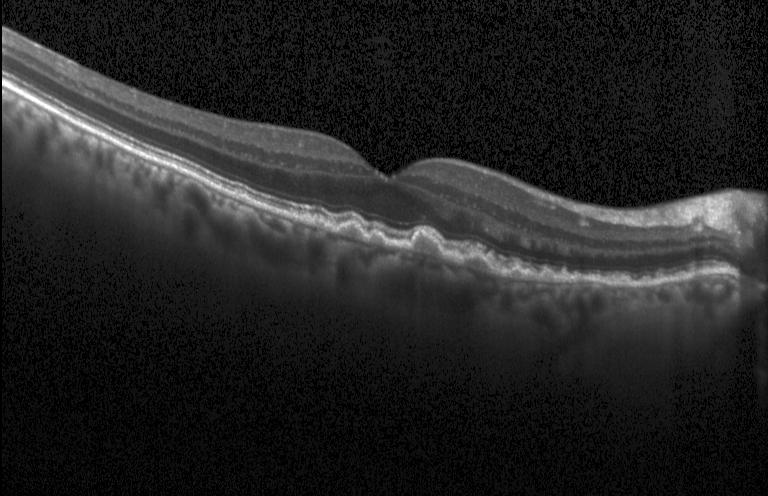

Optical coherence tomography B-scan; spectral-domain OCT; acquired on a Heidelberg Spectralis — OCT finding: drusen.